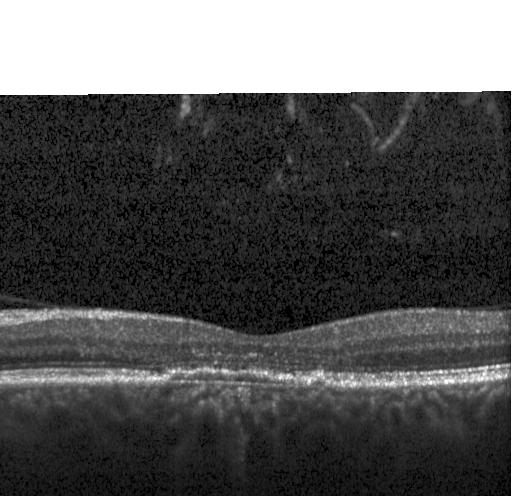

Impression: choroidal neovascularization.